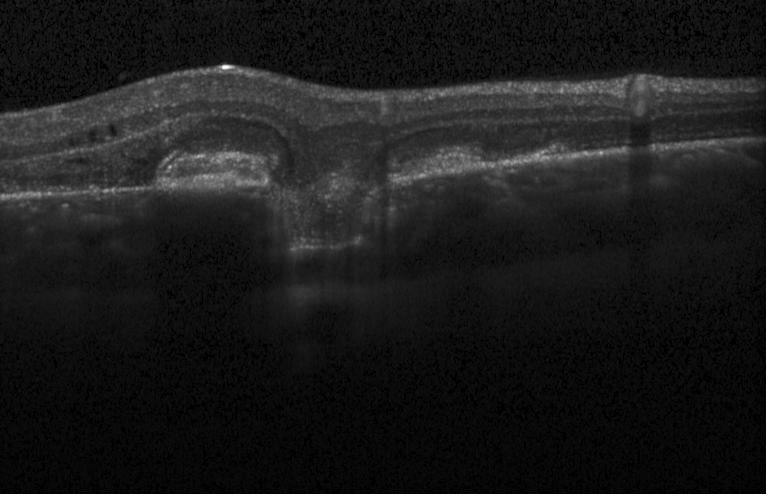
Heidelberg Spectralis. Retinal OCT B-scan. A choroidal neovascular membrane.